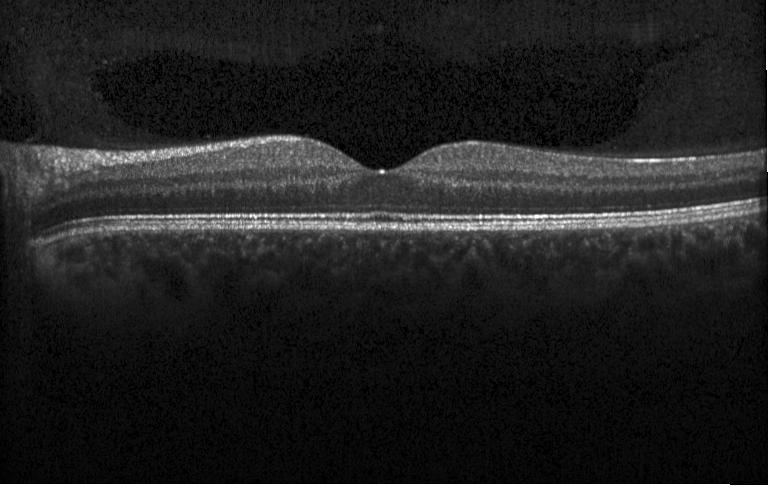 Finding: no choroidal neovascularization, no diabetic macular edema, and no drusen.